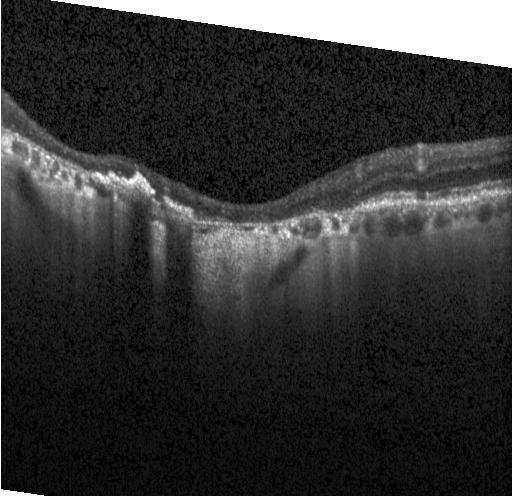
Retinal OCT cross-section · spectral-domain optical coherence tomography · horizontal scan through the fovea · Heidelberg Spectralis OCT system. The scan shows choroidal neovascularization.